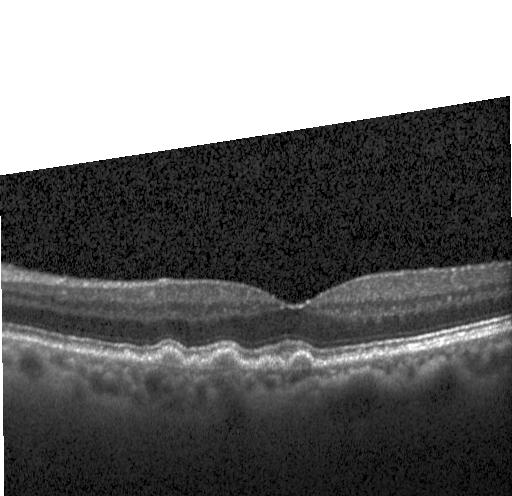

Optical coherence tomography B-scan — Dx: sub-RPE drusenoid deposits.